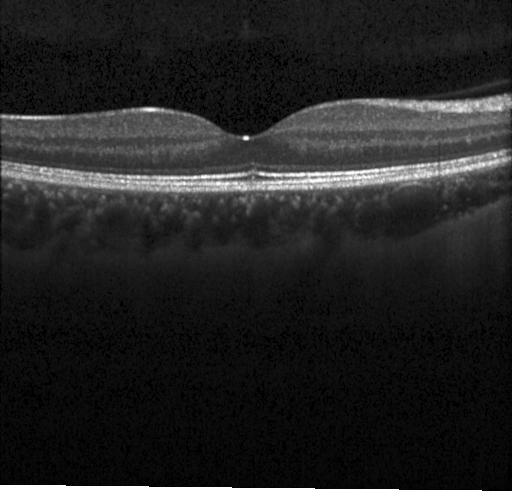
This B-scan demonstrates no evidence of choroidal neovascularization, diabetic macular edema, or drusen.